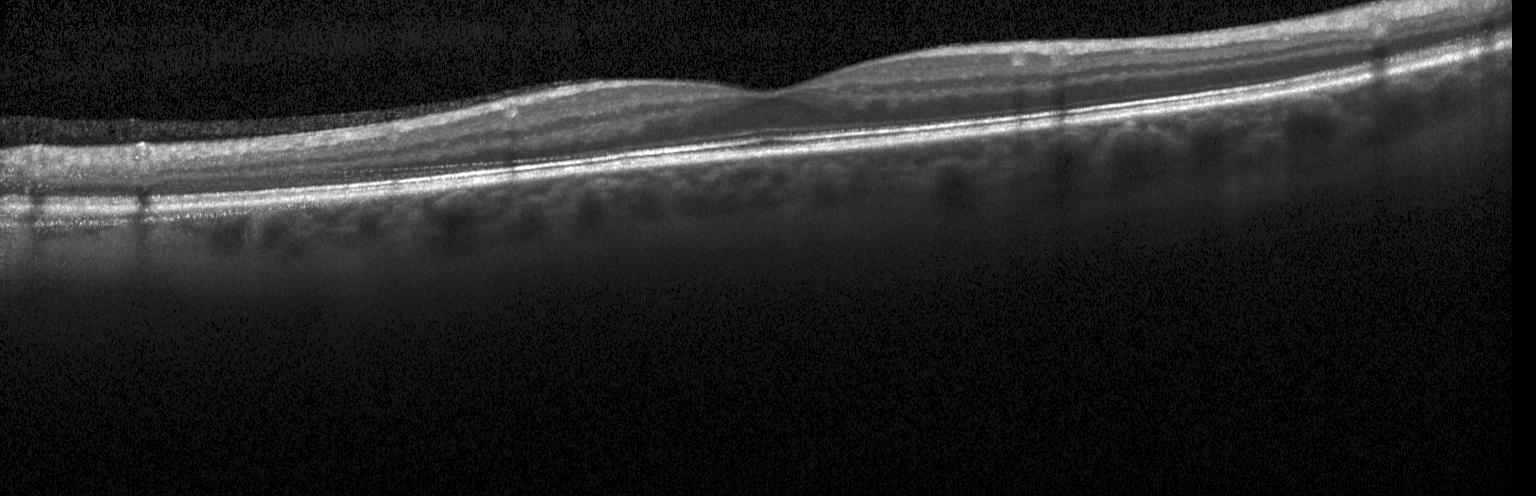

Optical coherence tomography B-scan
Impression: no evidence of choroidal neovascularization, diabetic macular edema, or drusen.